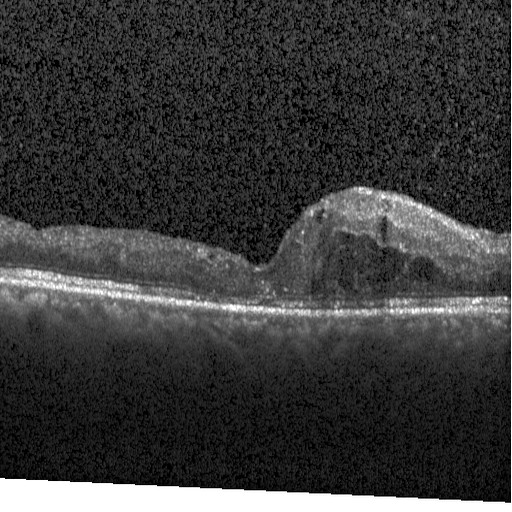

OCT scan showing diabetic macular edema (DME).